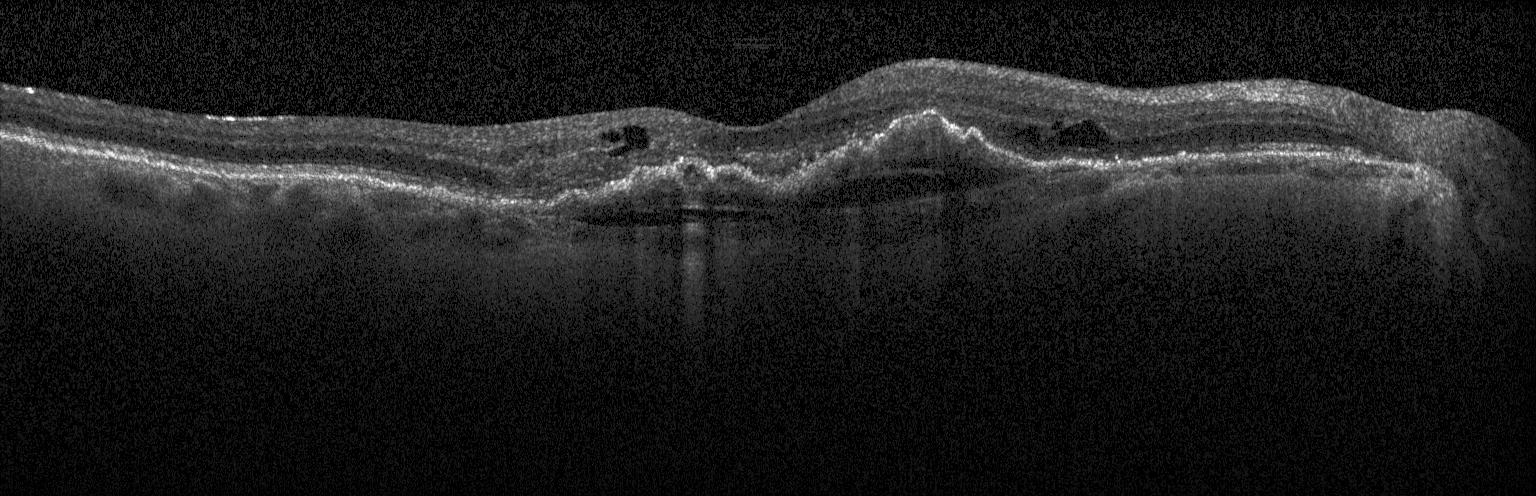 Optical coherence tomography B-scan
Finding: a choroidal neovascular membrane.